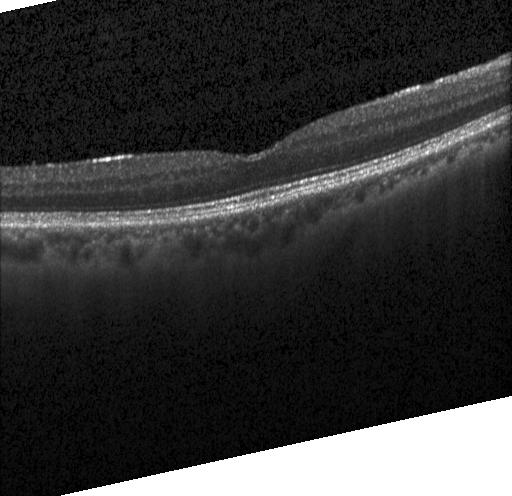 Impression: no choroidal neovascularization, no diabetic macular edema, and no drusen.